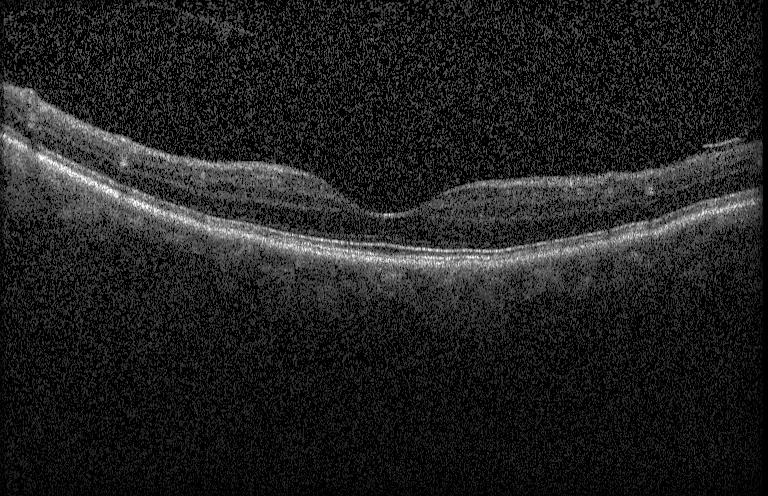
OCT finding: no evidence of choroidal neovascularization, diabetic macular edema, or drusen.